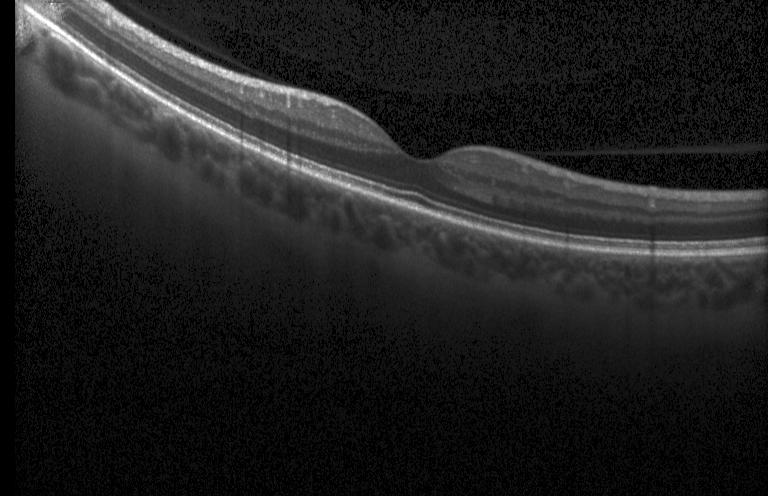
Macular OCT: no evidence of choroidal neovascularization, diabetic macular edema, or drusen.